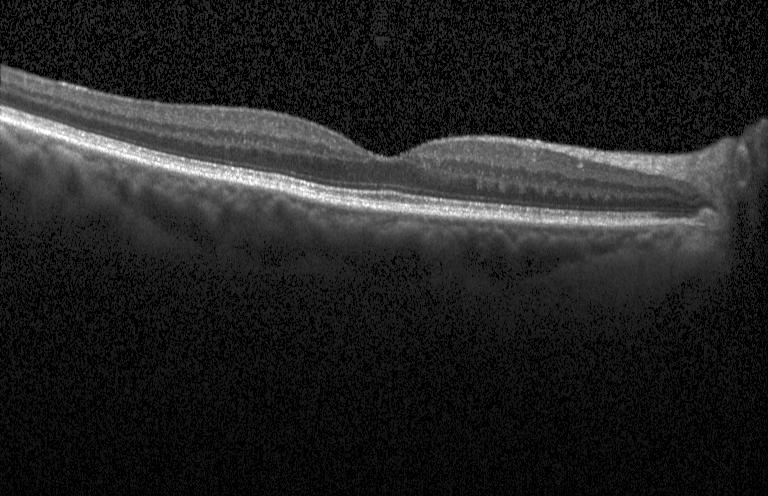 Optical coherence tomography scan
Impression: no CNV, no DME, and no drusen.